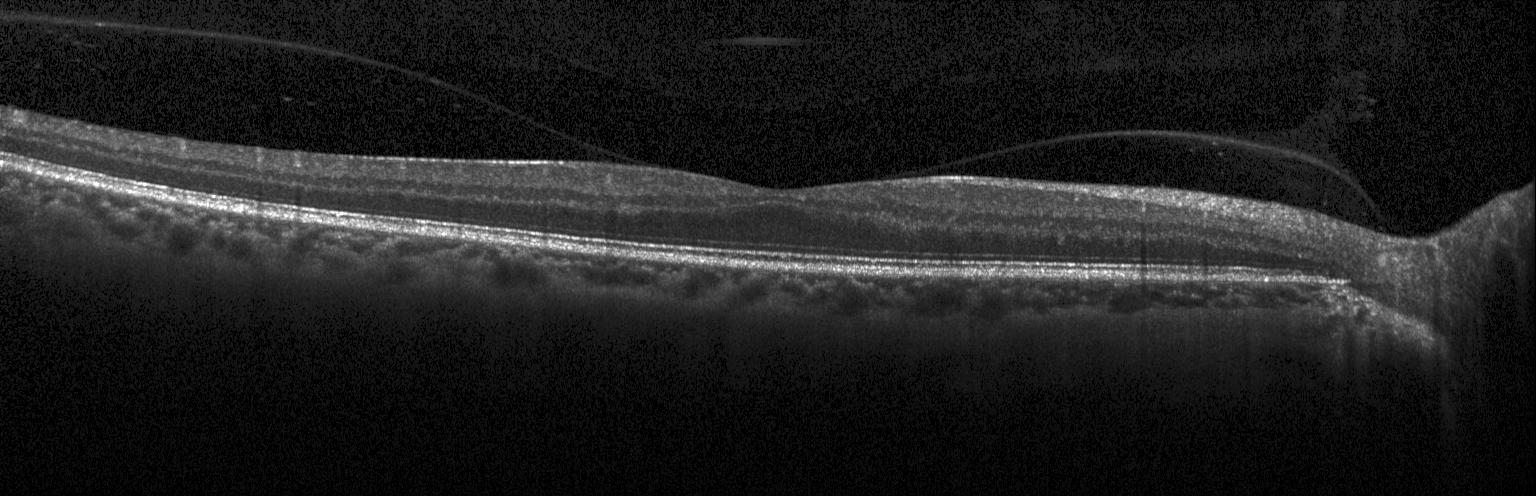
Finding: neither CNV, DME, nor drusen.